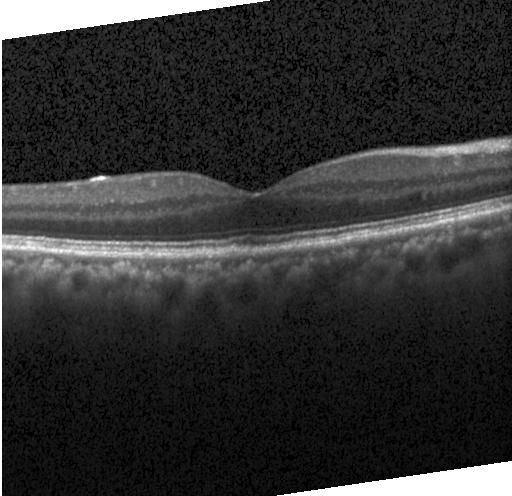
Macular scan. Spectral-domain OCT. Retinal OCT B-scan — Impression: no choroidal neovascularization, no diabetic macular edema, and no drusen.